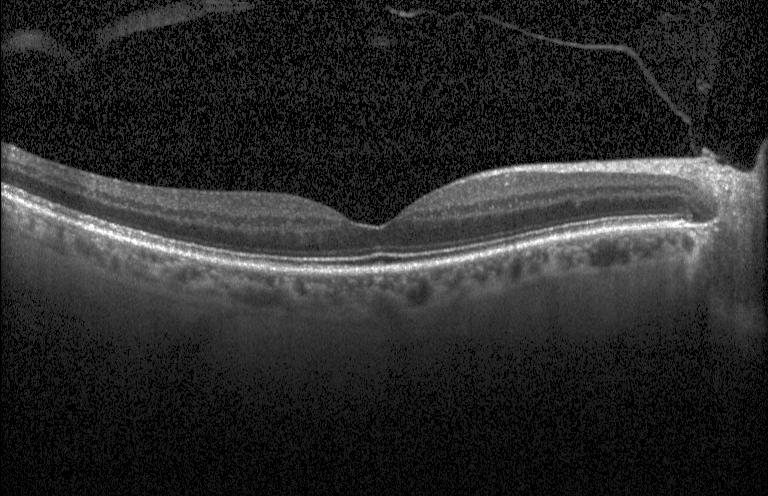

Impression: no evidence of choroidal neovascularization, diabetic macular edema, or drusen.